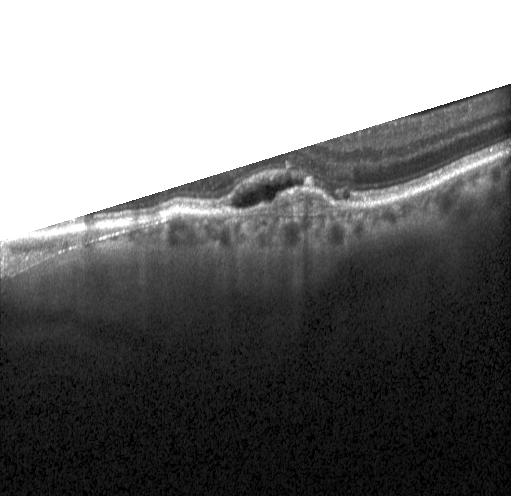
This B-scan demonstrates CNV.